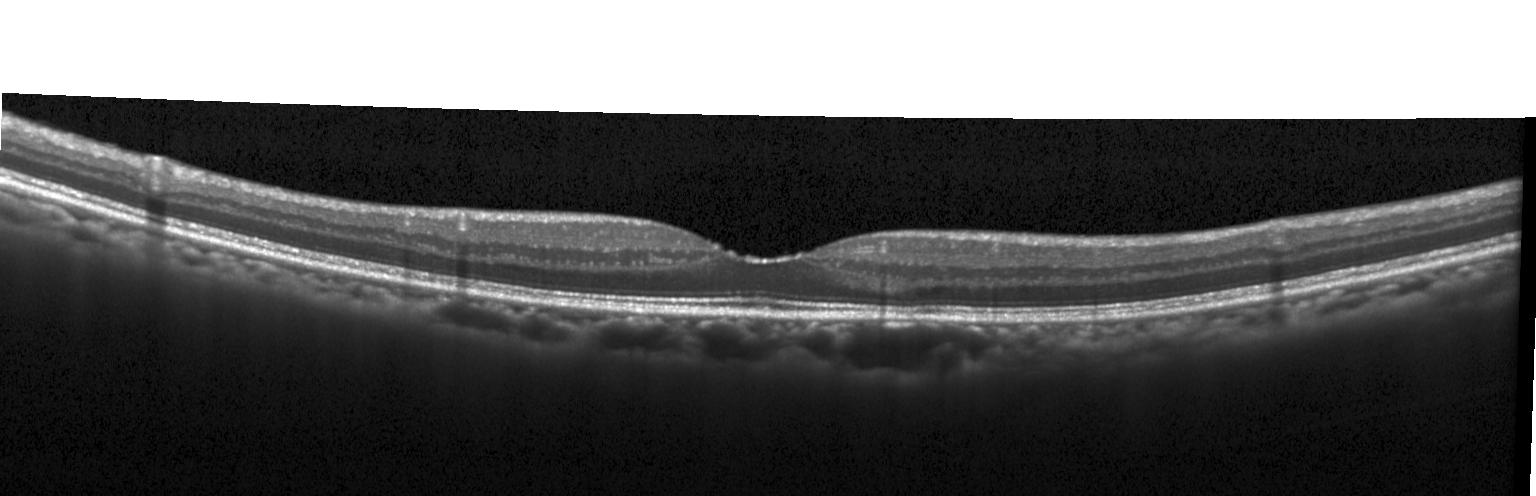 Optical coherence tomography scan. Diagnosis: no evidence of choroidal neovascularization, diabetic macular edema, or drusen.